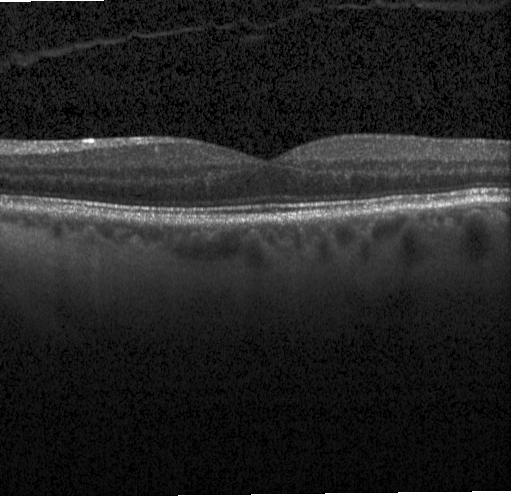

Macular OCT: neither choroidal neovascularization, diabetic macular edema, nor drusen.